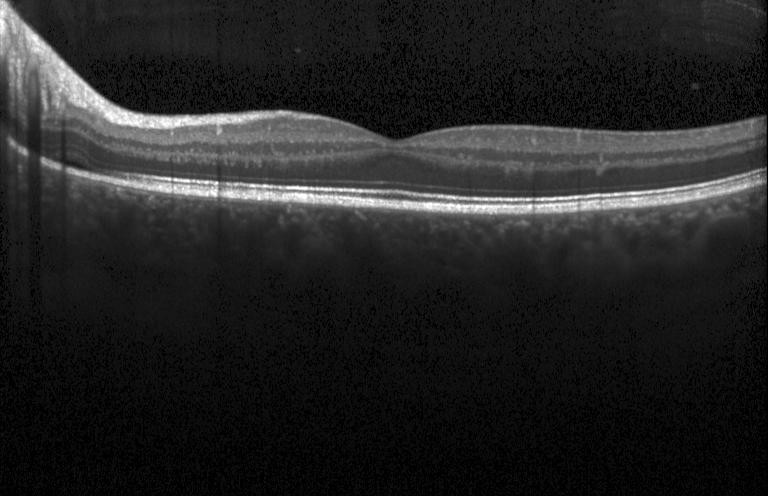

This B-scan demonstrates no choroidal neovascularization, diabetic macular edema, or drusen.